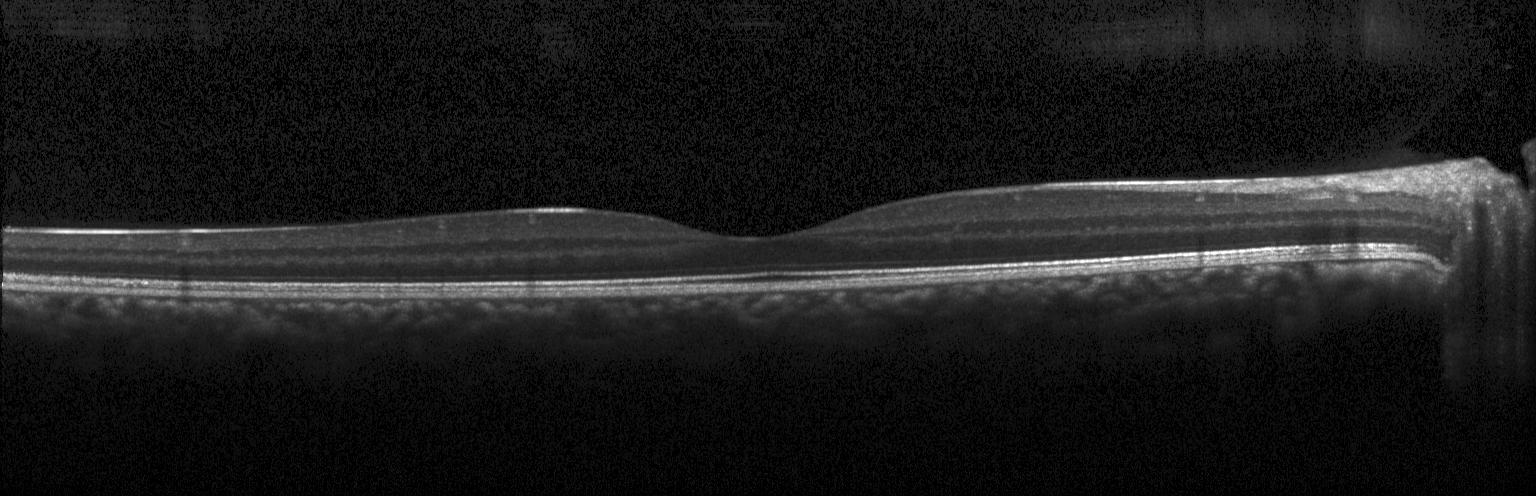
OCT B-scan · spectral-domain OCT · Heidelberg Spectralis · macular scan.
Neither CNV, DME, nor drusen.